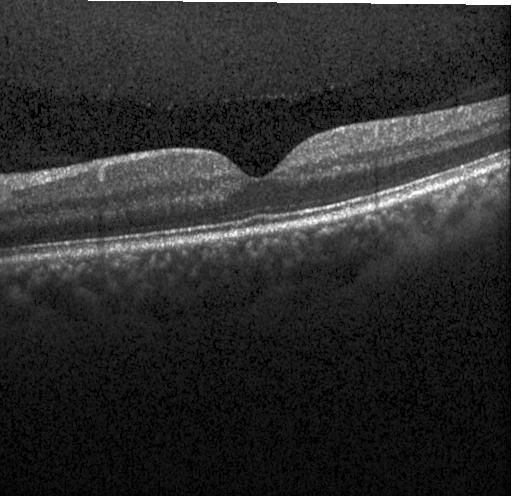

Acquired on a Heidelberg Spectralis · OCT B-scan — The scan shows no evidence of CNV, DME, or drusen.